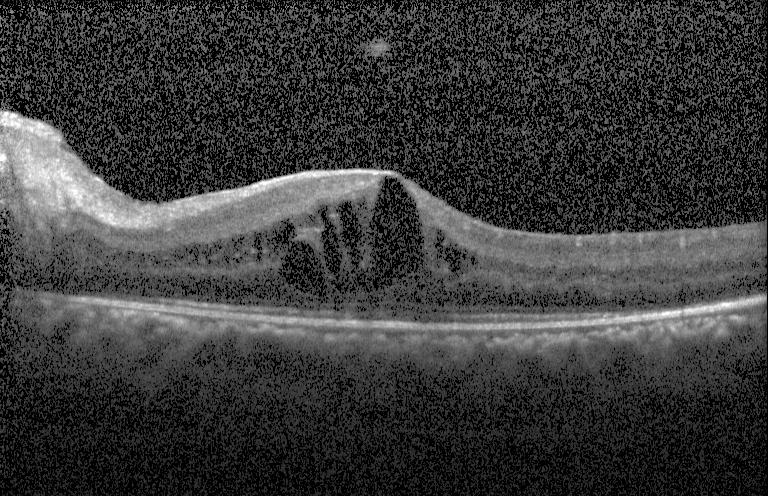
Spectral-domain OCT B-scan: diabetic macular edema (DME).